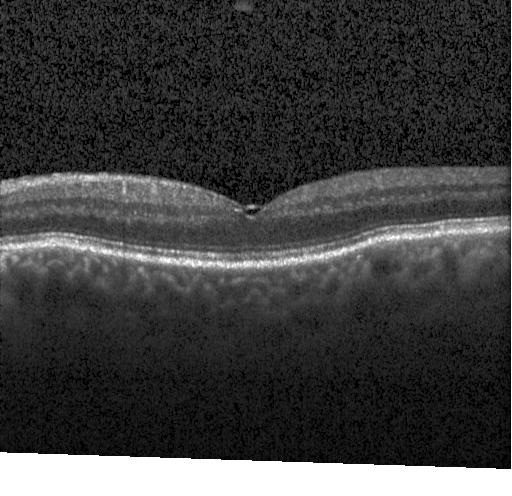

Dx: no choroidal neovascularization, diabetic macular edema, or drusen.